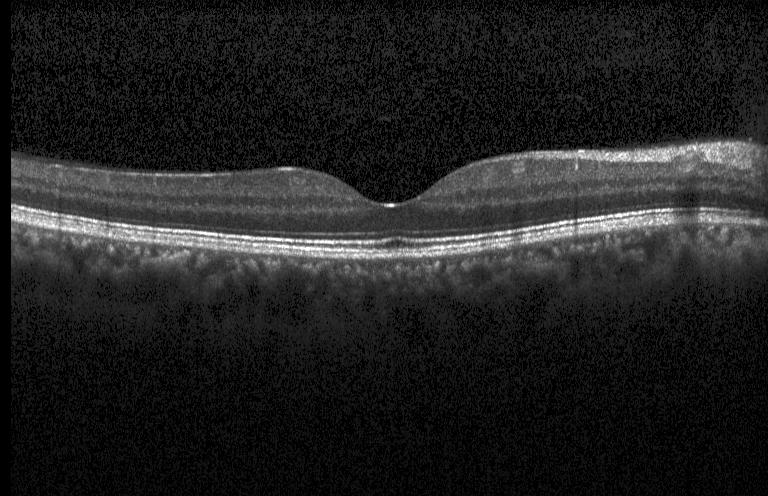

Optical coherence tomography scan; through the macula.
The scan shows no choroidal neovascularization, no diabetic macular edema, and no drusen.